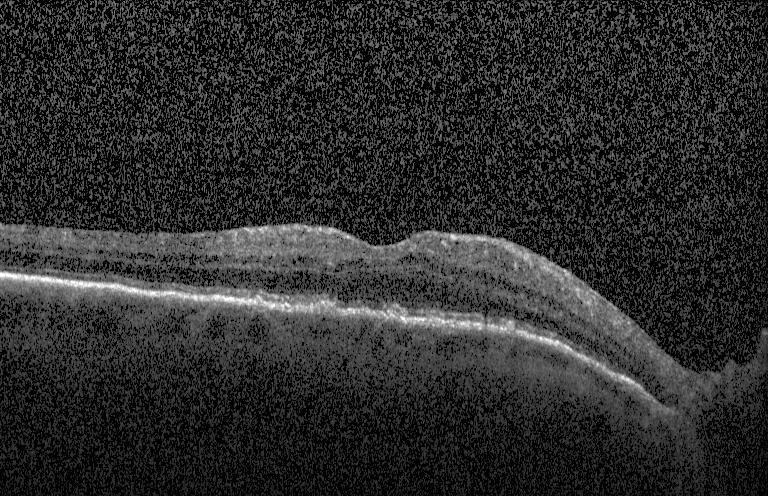

Acquired on a Heidelberg Spectralis, retinal OCT cross-section, through the macula
Finding: drusen.